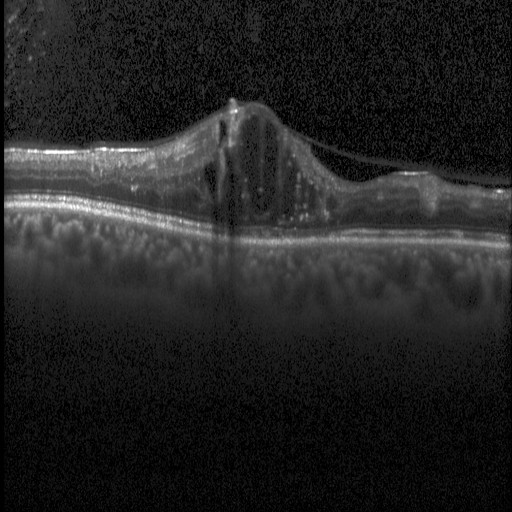

Diagnosis: diabetic macular edema (DME).